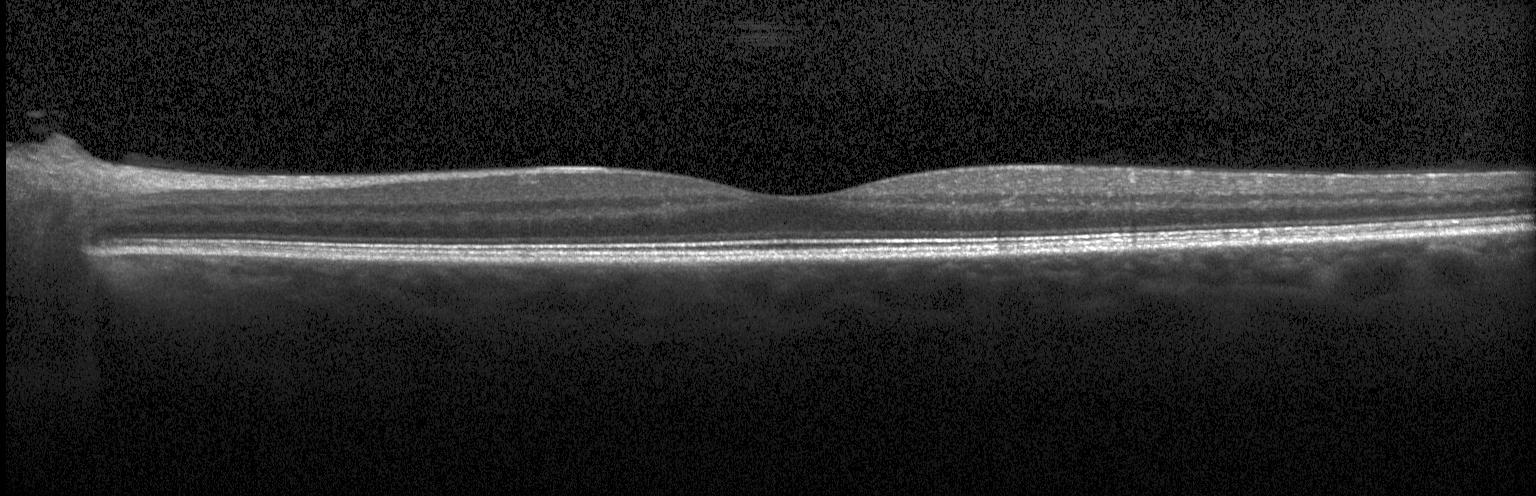

OCT B-scan · spectral-domain optical coherence tomography · fovea-centered
Macular OCT: no evidence of choroidal neovascularization, diabetic macular edema, or drusen.